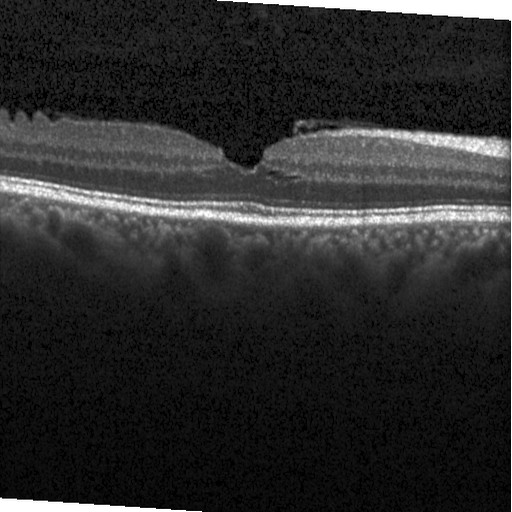
The scan shows diabetic macular edema.